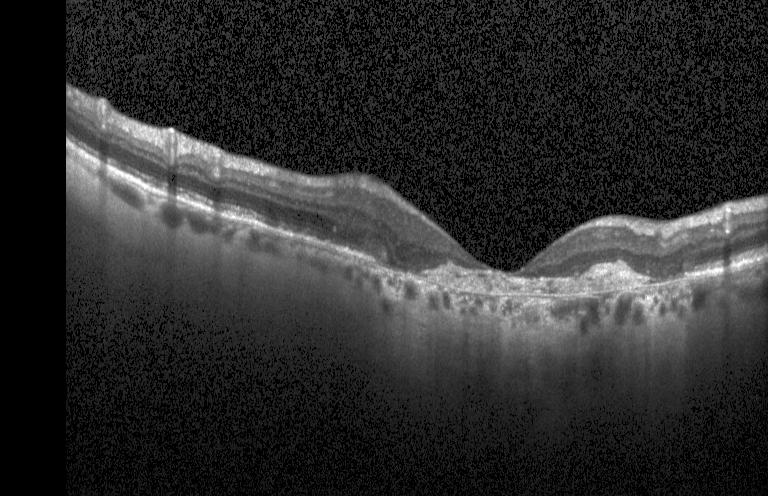 Diagnosis: a choroidal neovascular membrane.